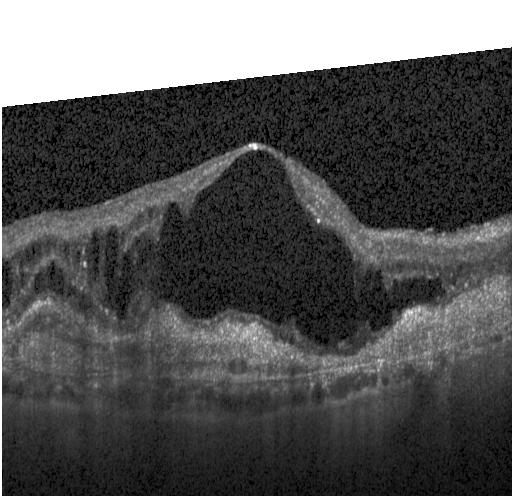
Retinal OCT B-scan; spectral-domain optical coherence tomography; Heidelberg Spectralis OCT system; macular scan
Dx: choroidal neovascularization (CNV).